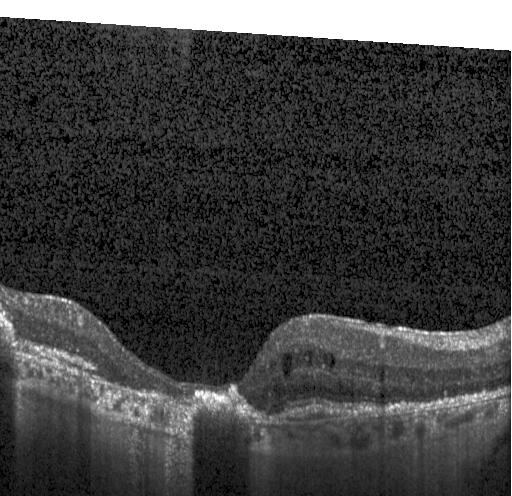
Retinal OCT B-scan
Choroidal neovascularization.